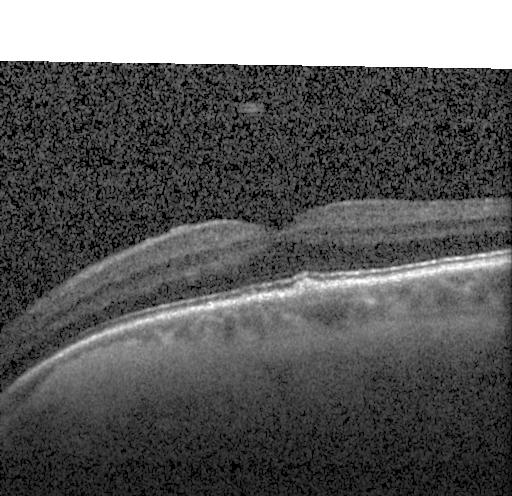

Dx: sub-RPE drusenoid deposits.